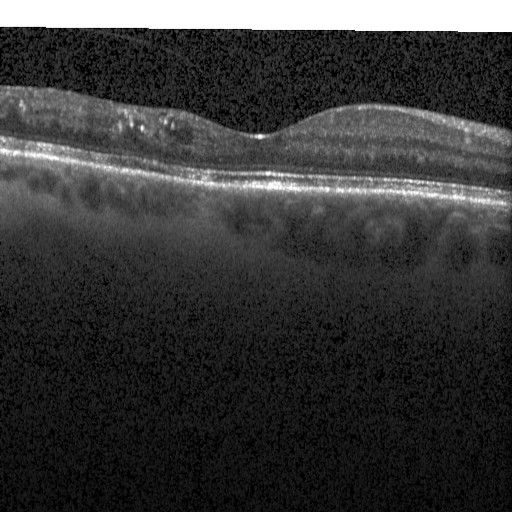
Horizontal scan through the fovea; Heidelberg Spectralis OCT system; spectral-domain optical coherence tomography; retinal OCT cross-section.
OCT finding: diabetic macular edema (DME).